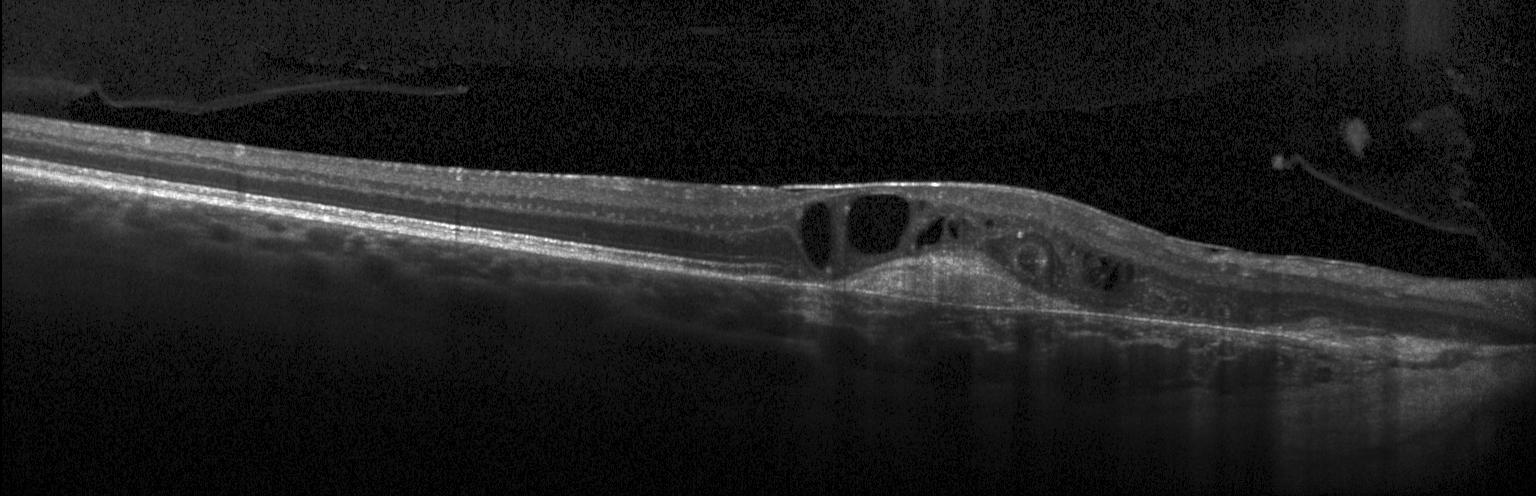
OCT line scan
This B-scan demonstrates a choroidal neovascular membrane.